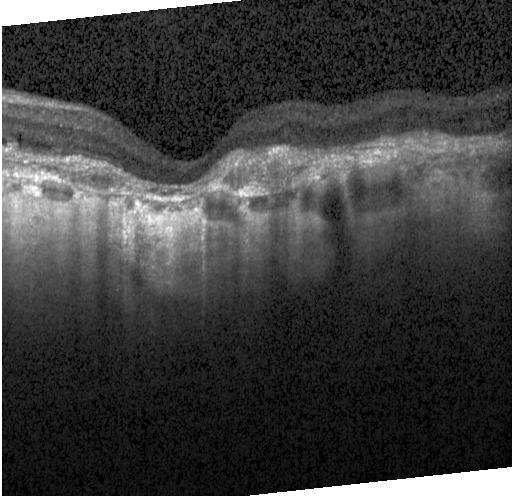 CNV.